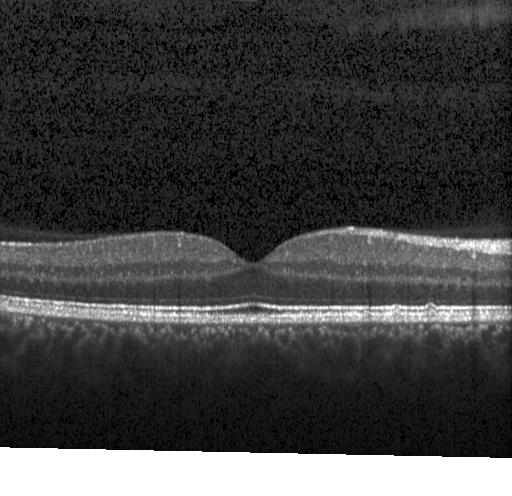 Through the macula. Heidelberg Spectralis. Retinal OCT B-scan. This B-scan demonstrates no CNV, no DME, and no drusen.